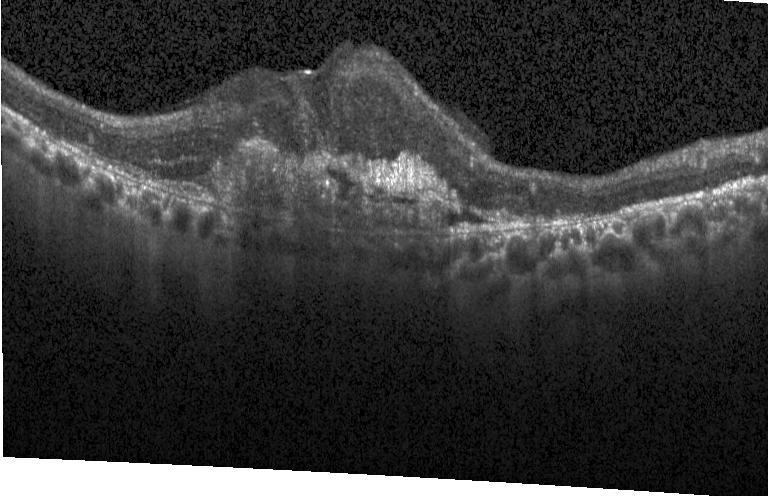
Spectral-domain OCT B-scan: CNV.